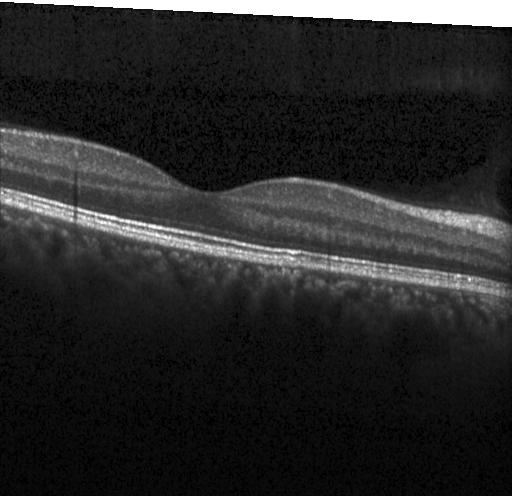 Diagnosis: no evidence of CNV, DME, or drusen.